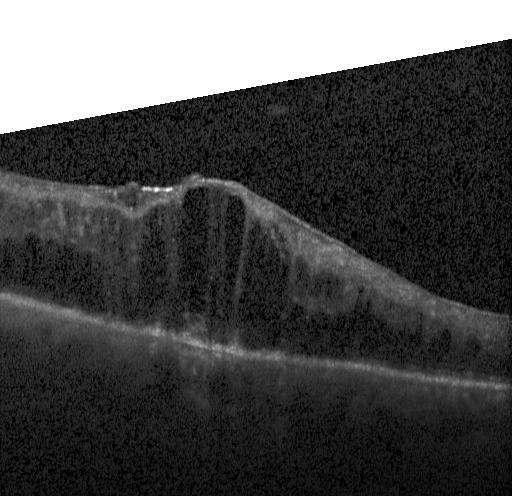 Instrument: Heidelberg Spectralis · optical coherence tomography B-scan · spectral-domain OCT
Finding: diabetic macular edema (DME).